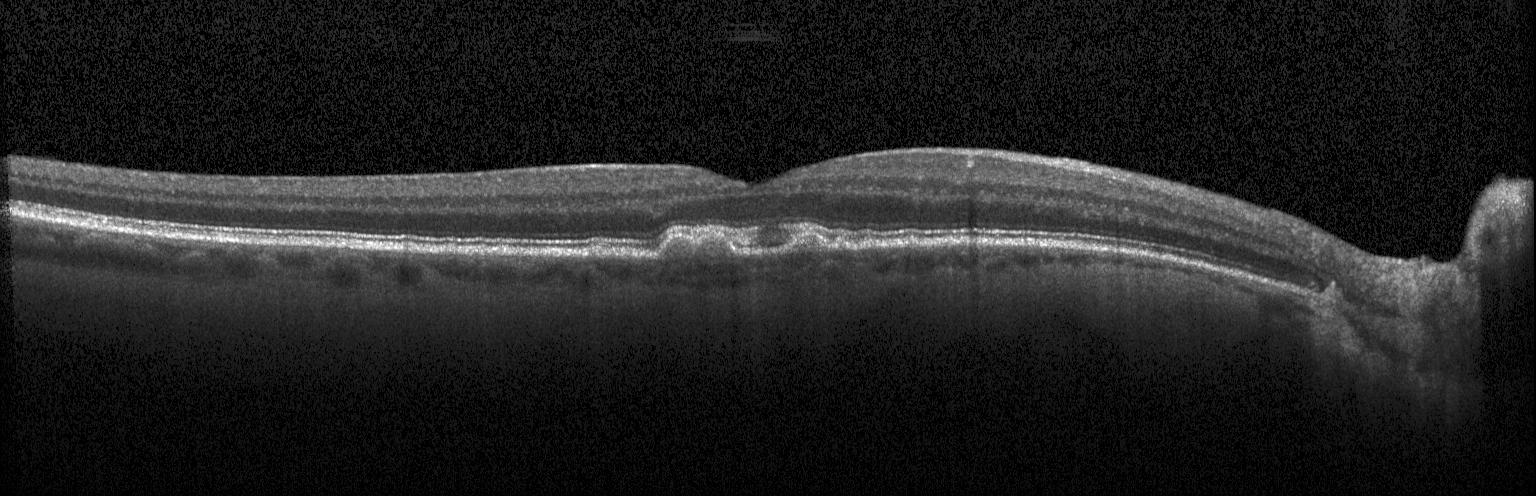 Instrument: Heidelberg Spectralis. Through the macula. SD-OCT. Optical coherence tomography B-scan. Diagnosis: sub-RPE drusenoid deposits.